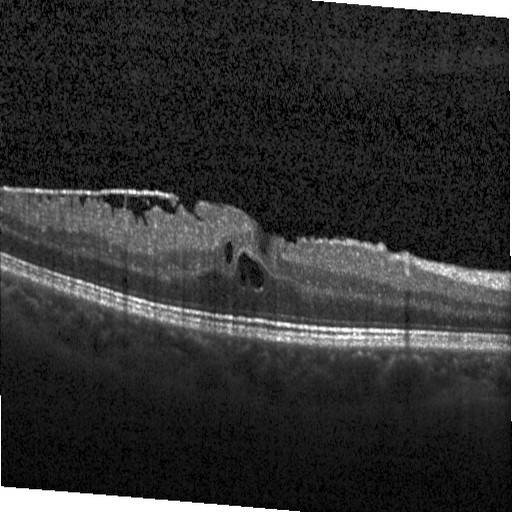

Fovea-centered · OCT line scan · spectral-domain optical coherence tomography. Finding: DME.